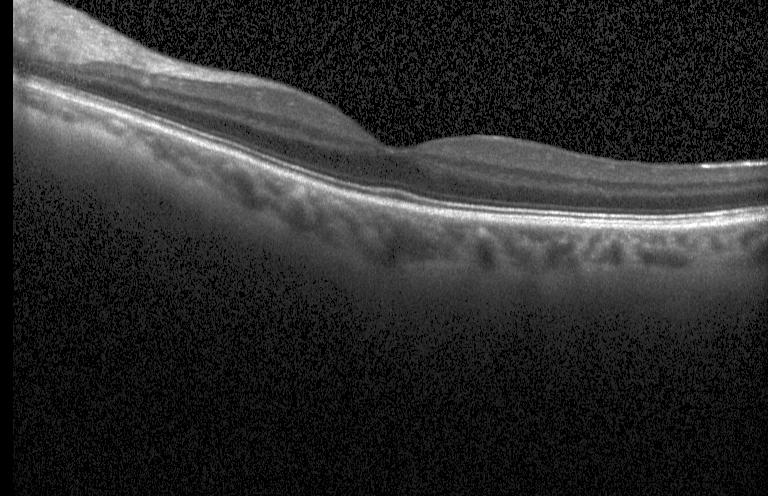
Retinal OCT cross-section. Macular scan — This B-scan demonstrates no choroidal neovascularization, diabetic macular edema, or drusen.